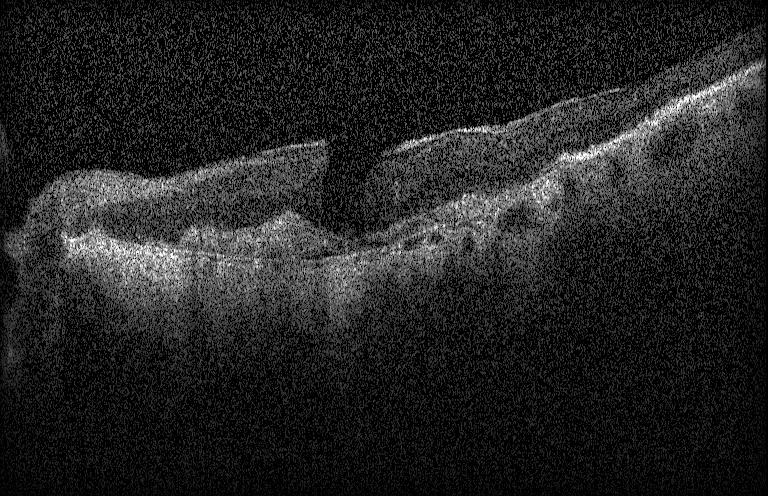
Dx: a choroidal neovascular membrane.